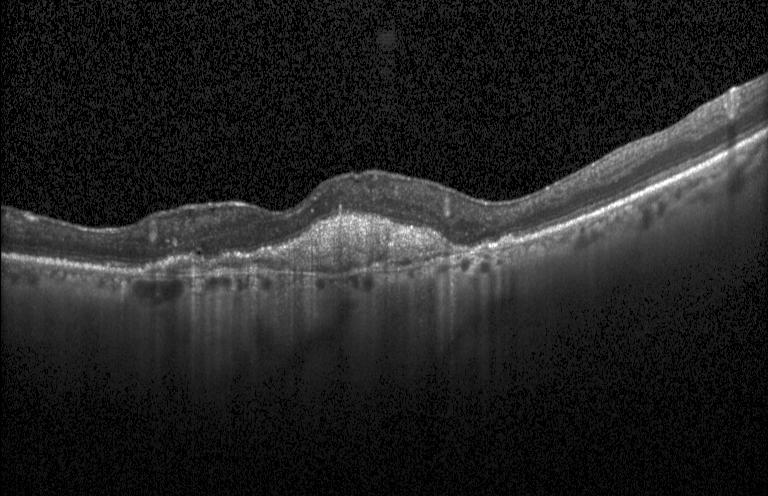

Impression: choroidal neovascularization.